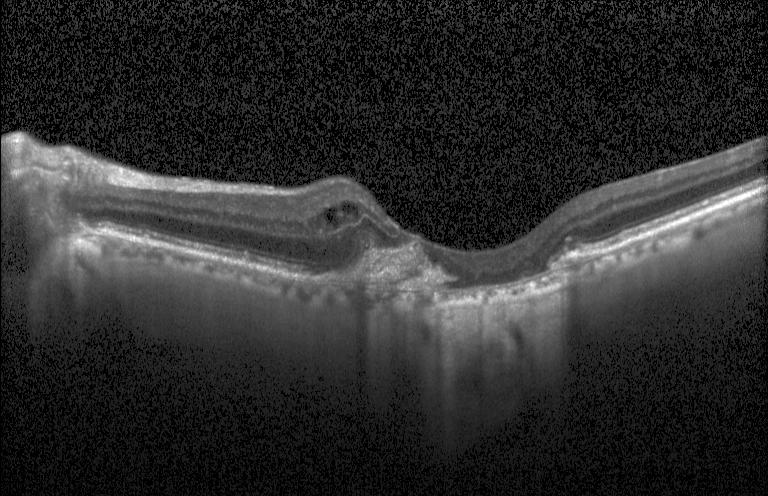
Optical coherence tomography scan · SD-OCT · acquired on a Heidelberg Spectralis — Diagnosis: a choroidal neovascular membrane.